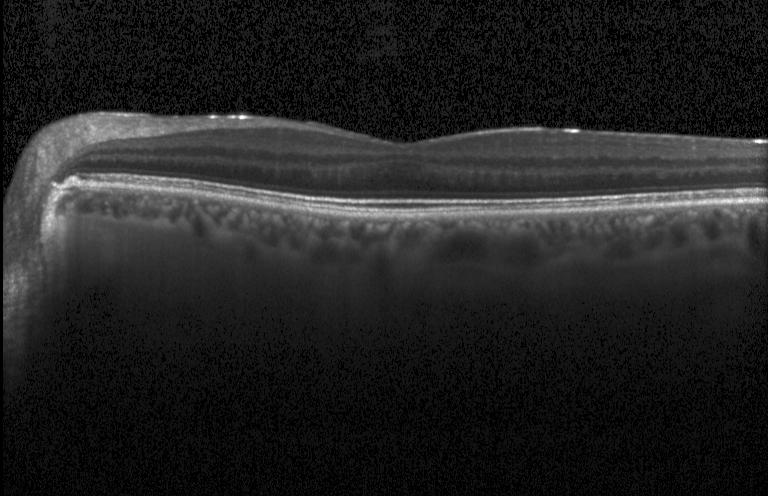
Impression: no evidence of CNV, DME, or drusen.